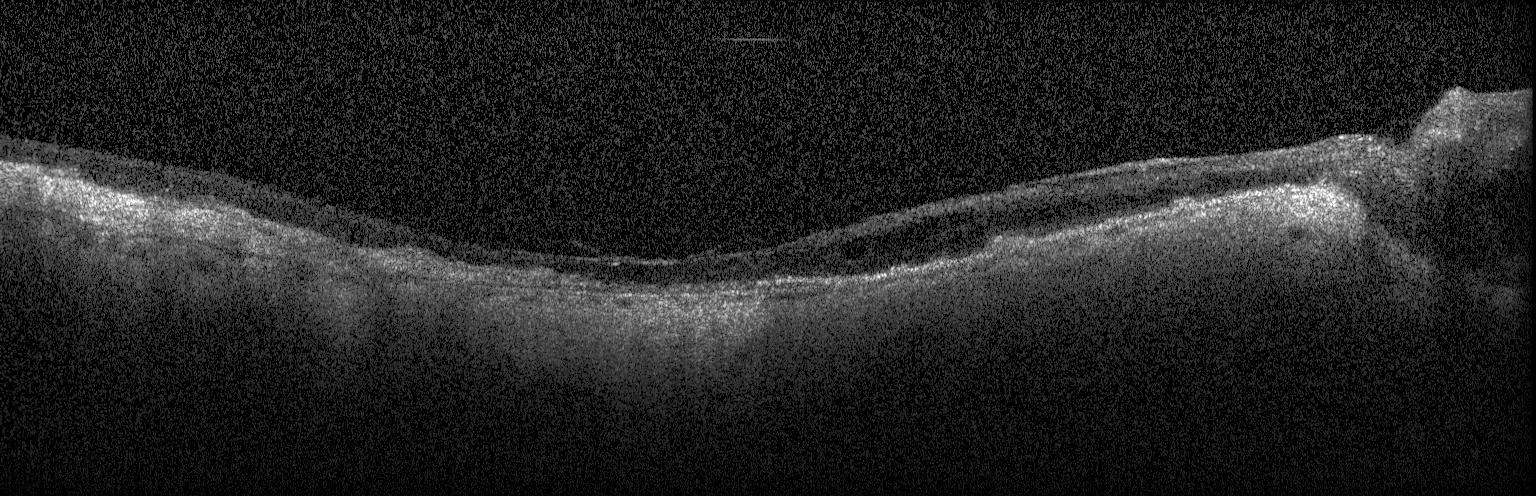 Optical coherence tomography B-scan — Finding: CNV.